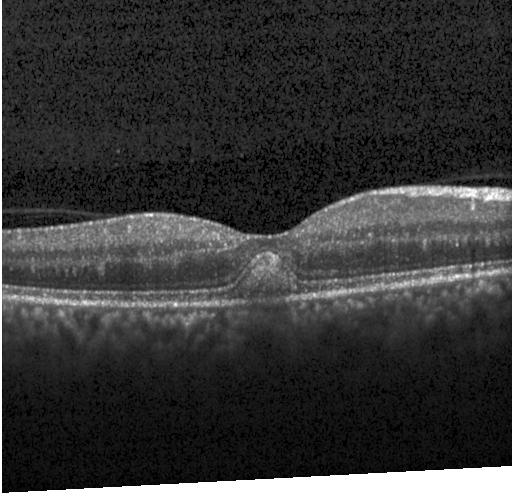
Optical coherence tomography B-scan — Finding: a choroidal neovascular membrane.